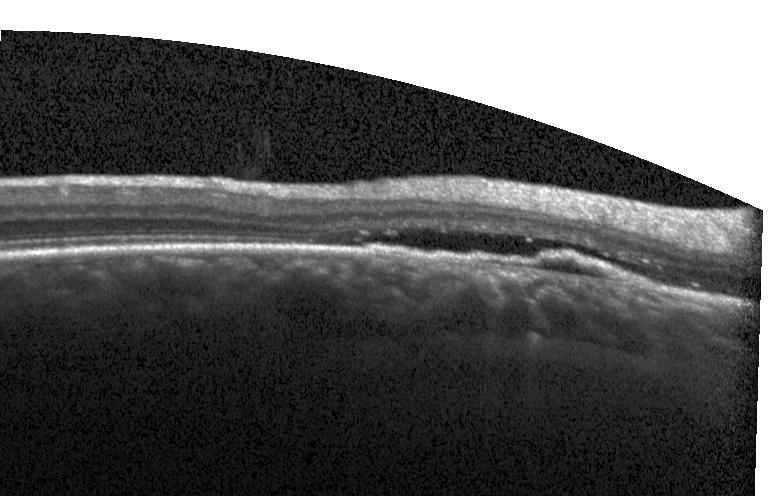 Macular scan · Heidelberg Spectralis · OCT B-scan
The scan shows CNV.